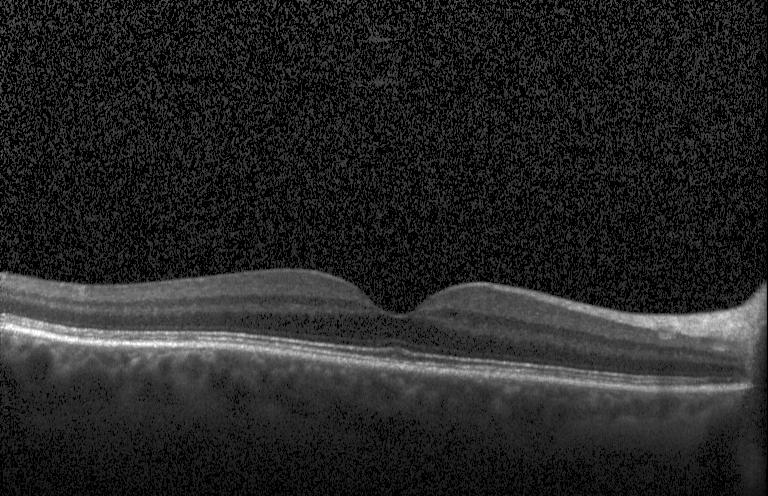

Optical coherence tomography B-scan
Impression: no evidence of choroidal neovascularization, diabetic macular edema, or drusen.